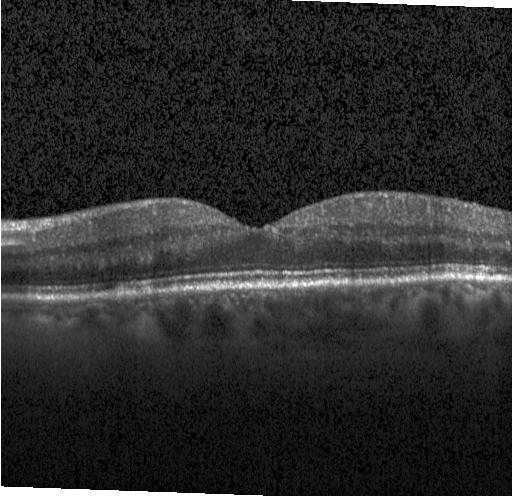 OCT line scan; acquired on a Heidelberg Spectralis; spectral-domain OCT; macular scan.
The scan shows no choroidal neovascularization, no diabetic macular edema, and no drusen.